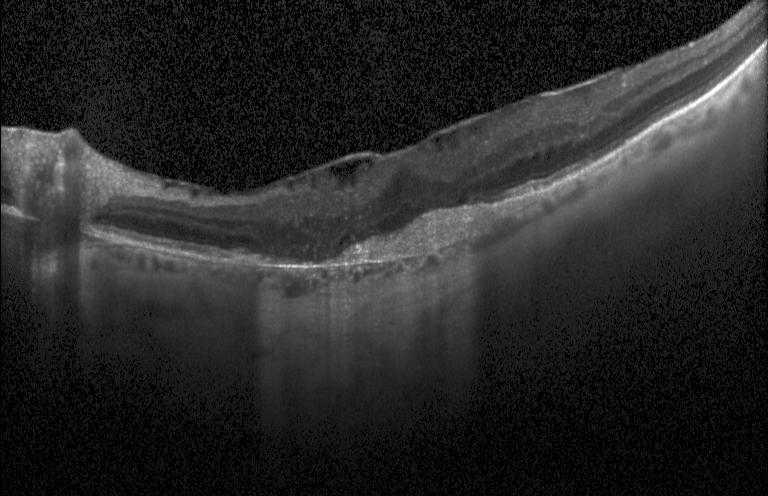
Optical coherence tomography B-scan — Finding: choroidal neovascularization.